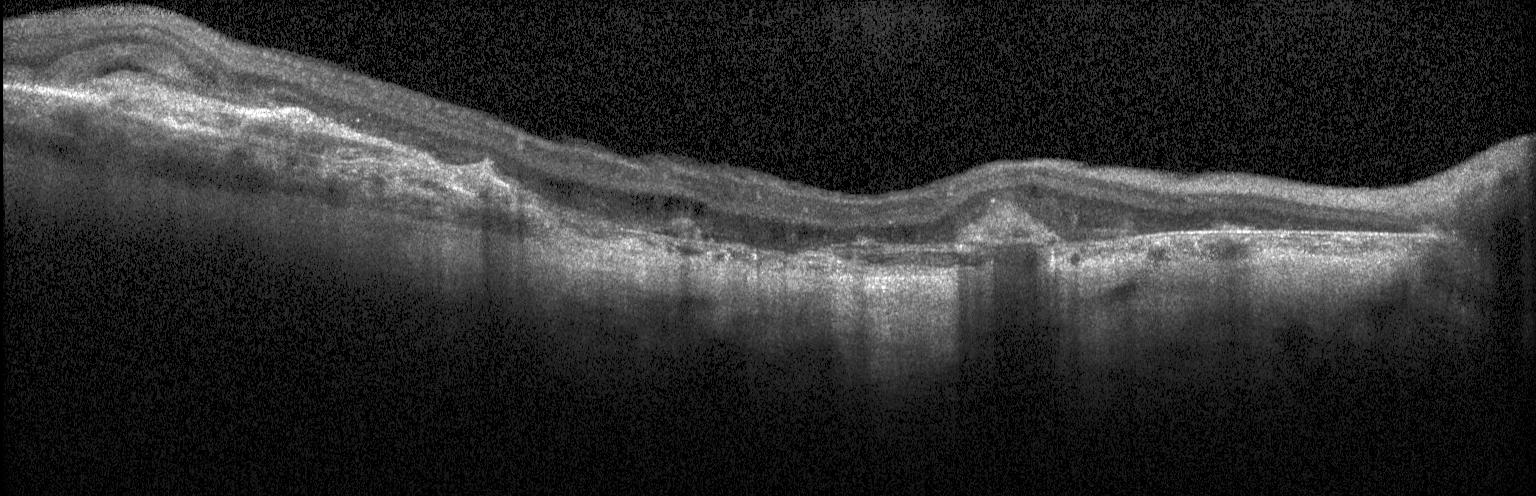 Impression: a choroidal neovascular membrane.